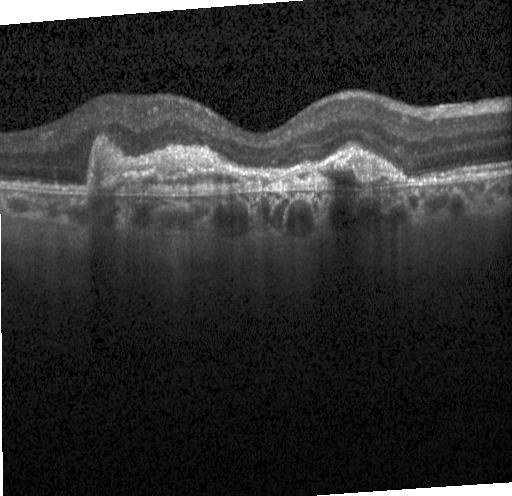
This B-scan demonstrates a choroidal neovascular membrane.